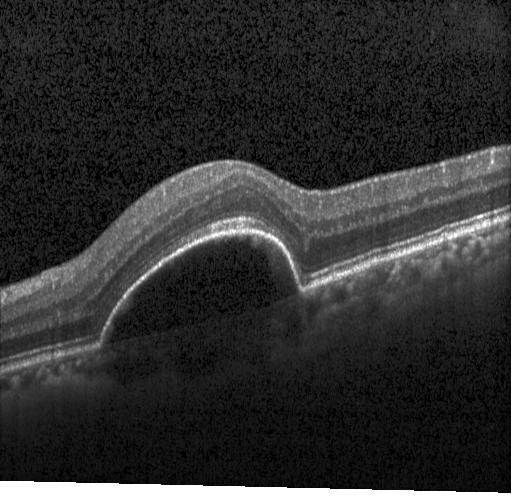 OCT B-scan. Spectral-domain OCT — The scan shows choroidal neovascularization.